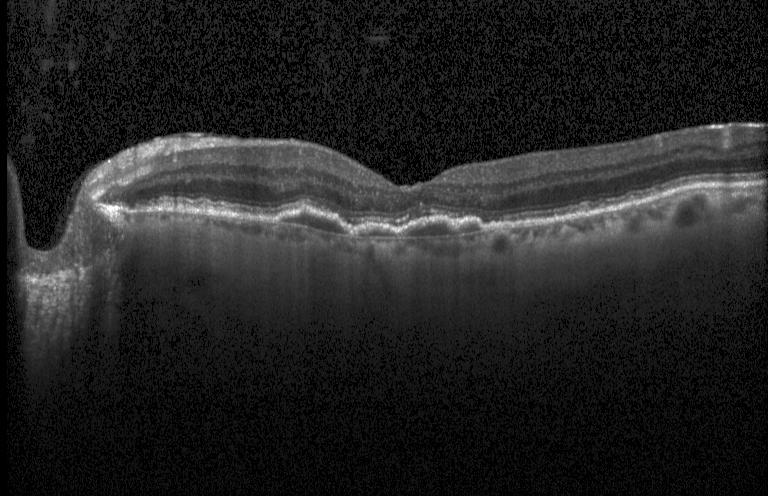

Optical coherence tomography scan; instrument: Heidelberg Spectralis.
Macular OCT: a choroidal neovascular membrane.